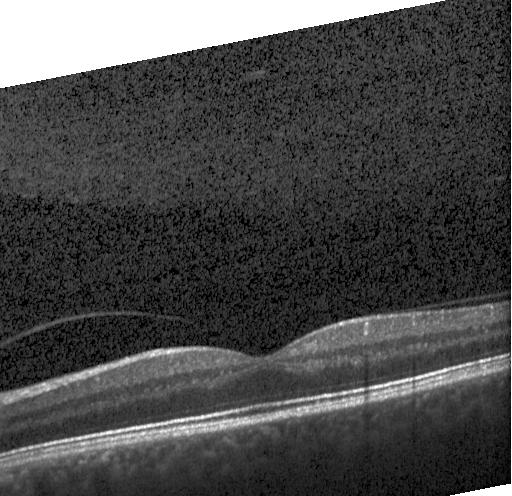 OCT B-scan — Finding: no evidence of CNV, DME, or drusen.